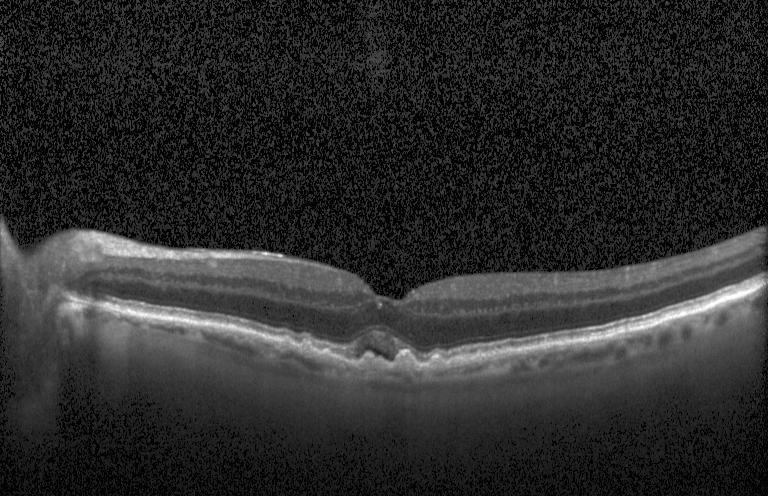

Retinal OCT B-scan
Finding: a choroidal neovascular membrane.